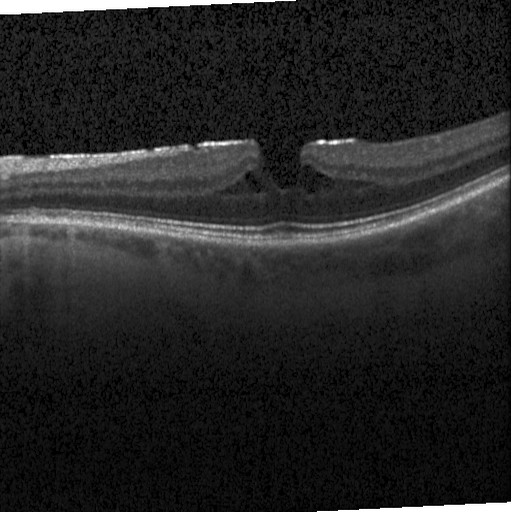
Fovea-centered; OCT B-scan.
Macular OCT: diabetic macular edema.